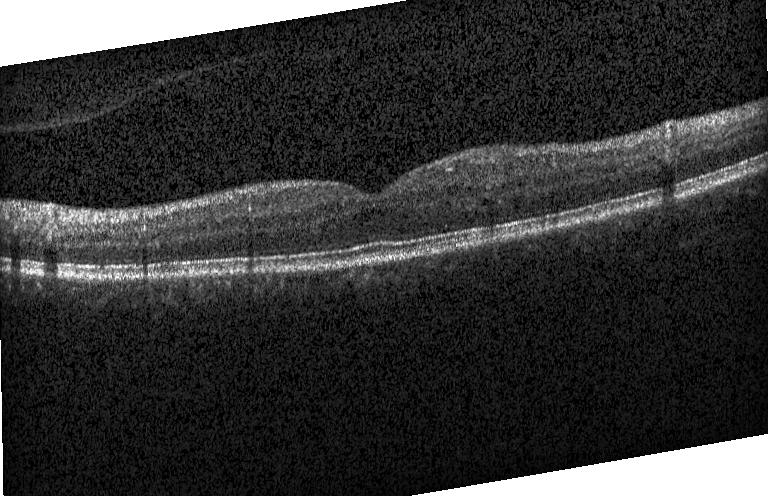 OCT finding: no choroidal neovascularization, diabetic macular edema, or drusen.